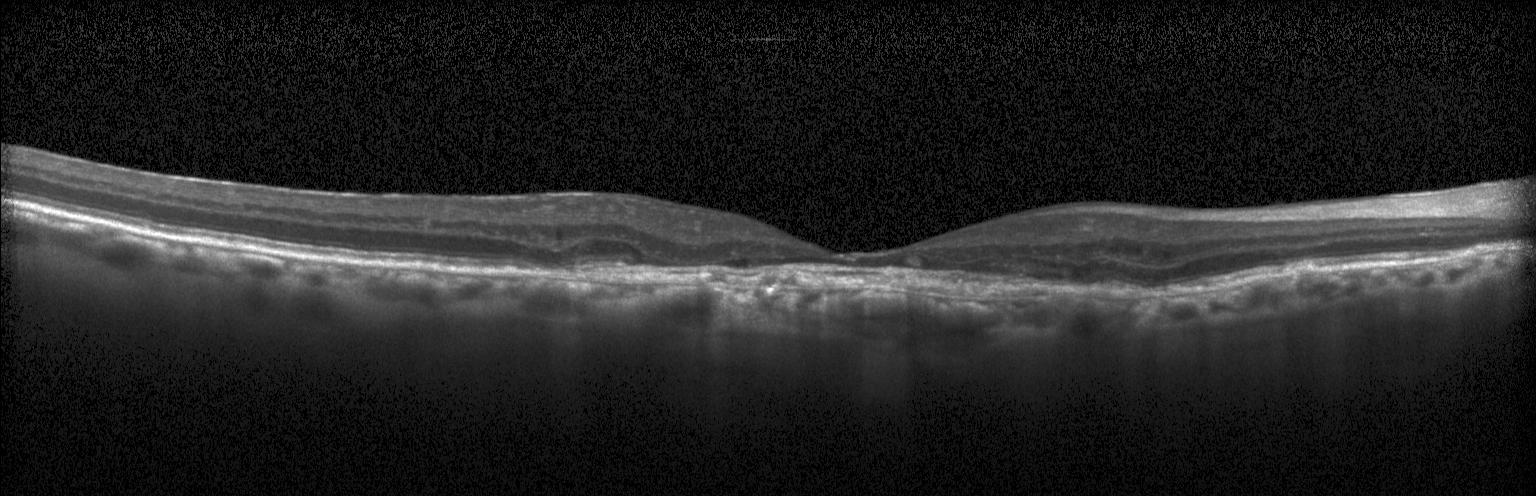 Instrument: Heidelberg Spectralis. OCT line scan.
Dx: a choroidal neovascular membrane.